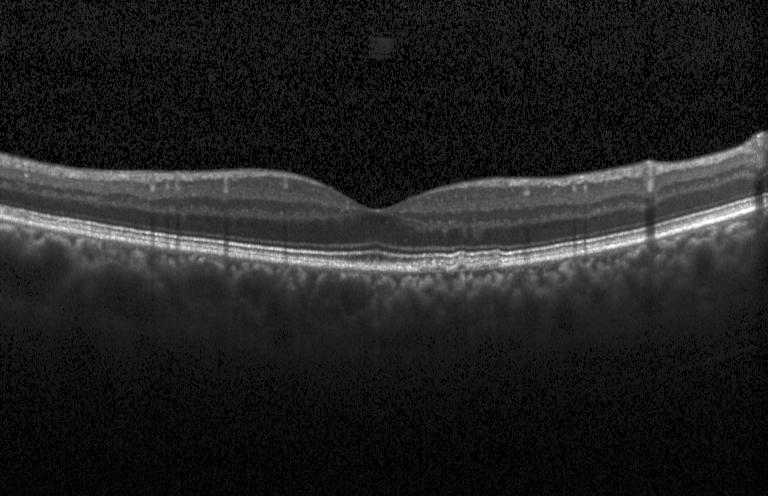

Diagnosis: multiple drusen.